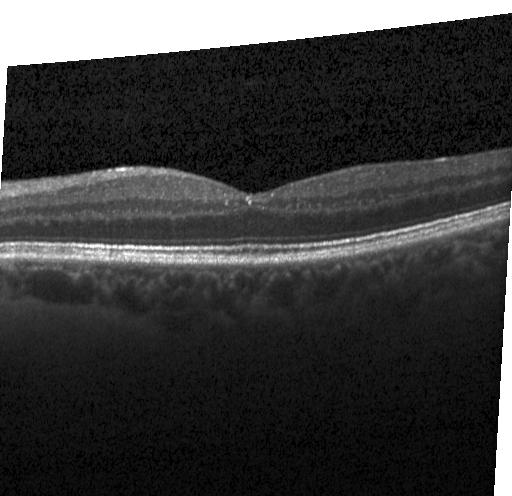

Impression: no CNV, DME, or drusen.